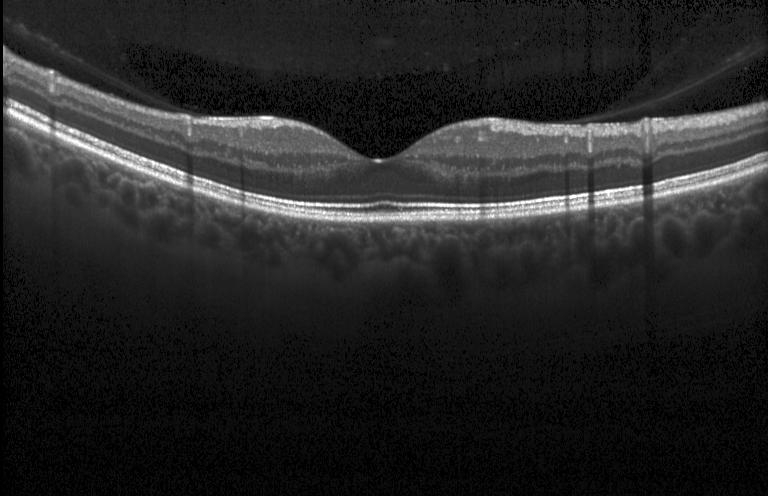
OCT scan showing no evidence of choroidal neovascularization, diabetic macular edema, or drusen.